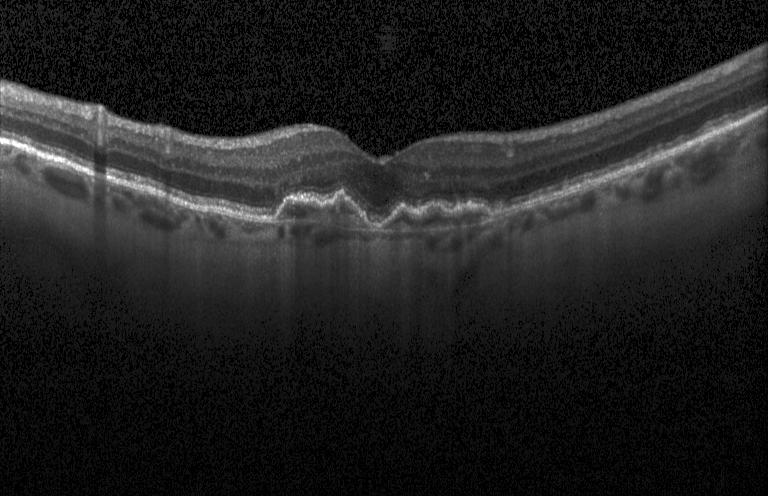

OCT B-scan showing choroidal neovascularization.